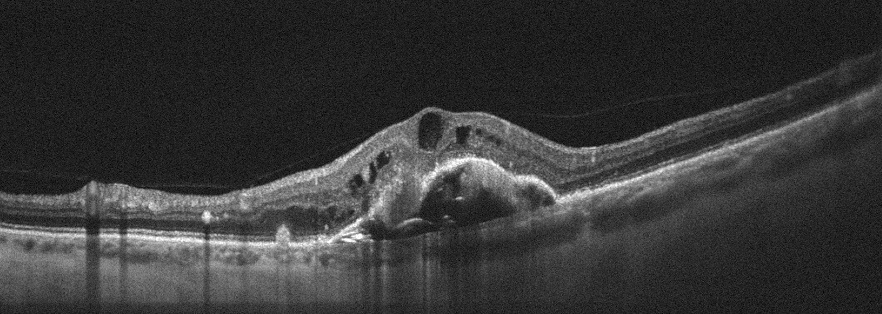
Acquired on an Optovue Avanti RTVue XR. OCT B-scan.
Finding: age-related macular degeneration.